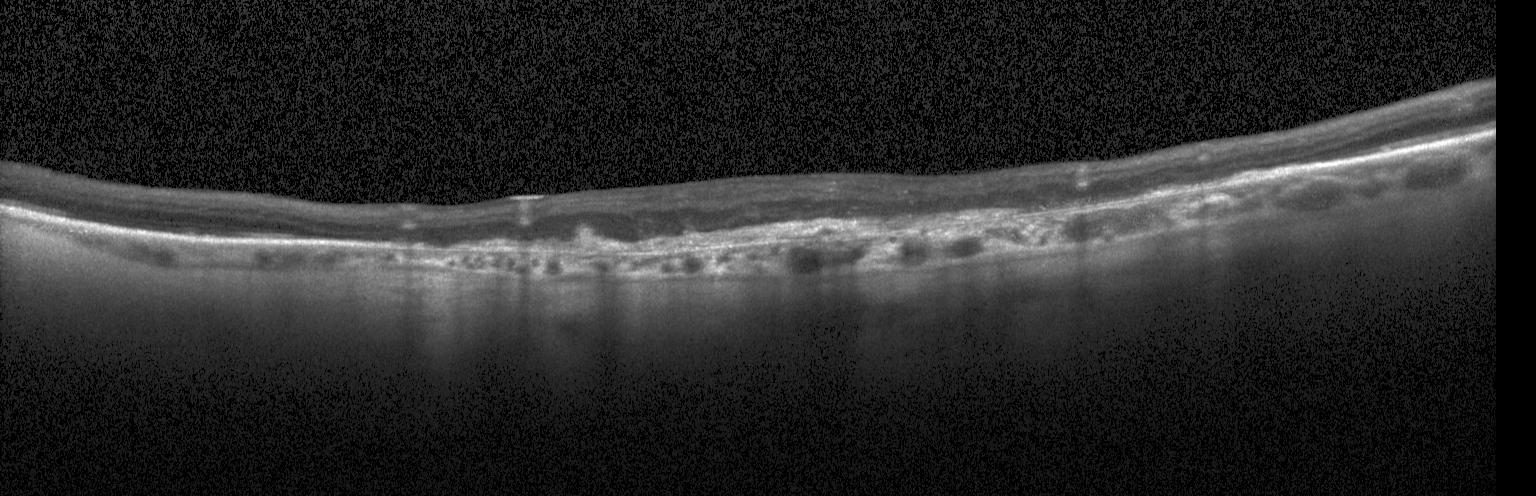 Optical coherence tomography B-scan · horizontal scan through the fovea.
This B-scan demonstrates a choroidal neovascular membrane.